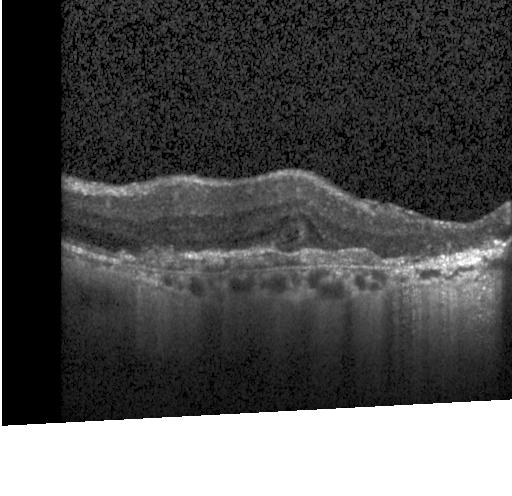 Acquired on a Heidelberg Spectralis · spectral-domain OCT · OCT B-scan · macular scan — Finding: CNV.